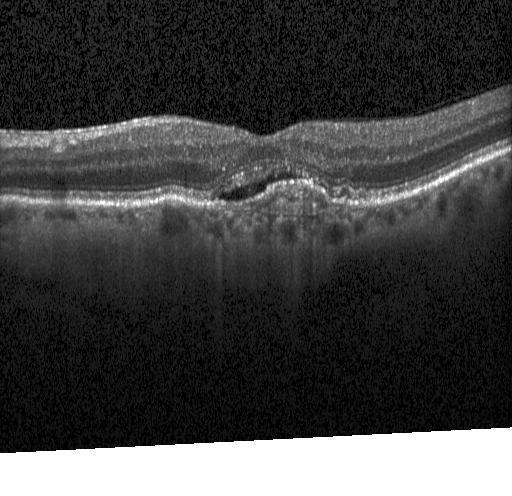
Spectral-domain optical coherence tomography, retinal OCT B-scan, horizontal scan through the fovea, instrument: Heidelberg Spectralis. Diagnosis: choroidal neovascularization (CNV).